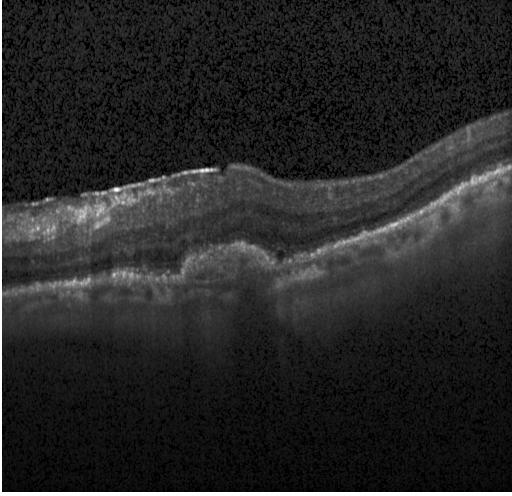 Instrument: Heidelberg Spectralis; through the macula; SD-OCT; OCT line scan
Assessment: choroidal neovascularization.